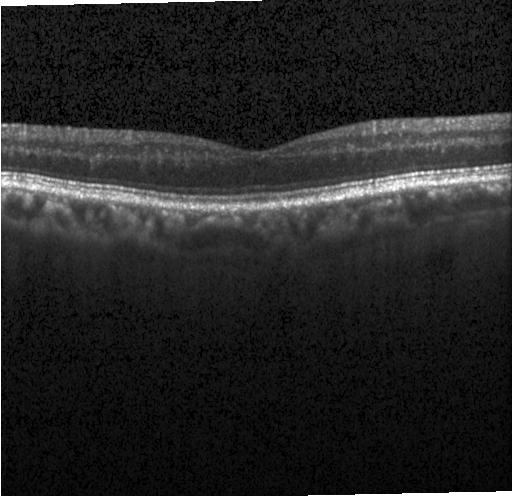 Macular scan. Spectral-domain optical coherence tomography. Optical coherence tomography scan. Heidelberg Spectralis — Finding: no evidence of CNV, DME, or drusen.